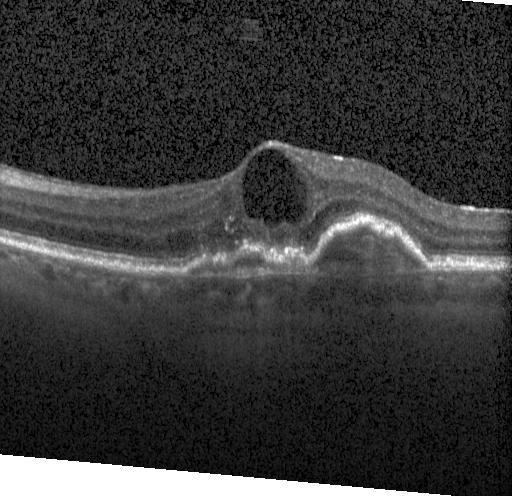
Spectral-domain OCT B-scan: a choroidal neovascular membrane.